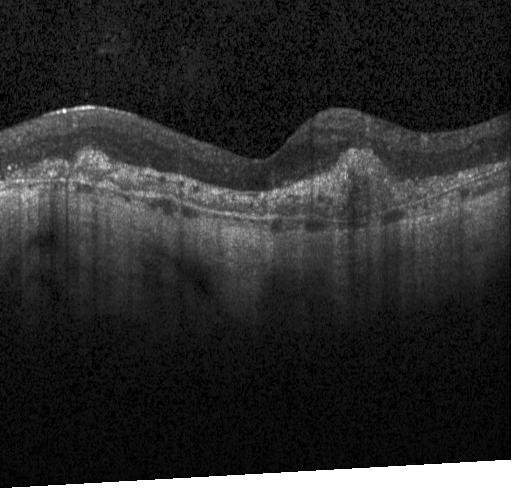

Horizontal scan through the fovea · Heidelberg Spectralis OCT system · optical coherence tomography B-scan.
Diagnosis: choroidal neovascularization.